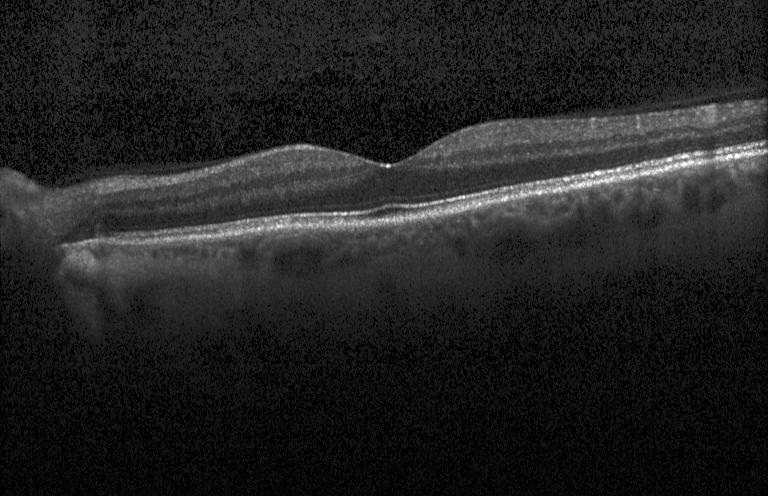
OCT finding: no CNV, no DME, and no drusen.